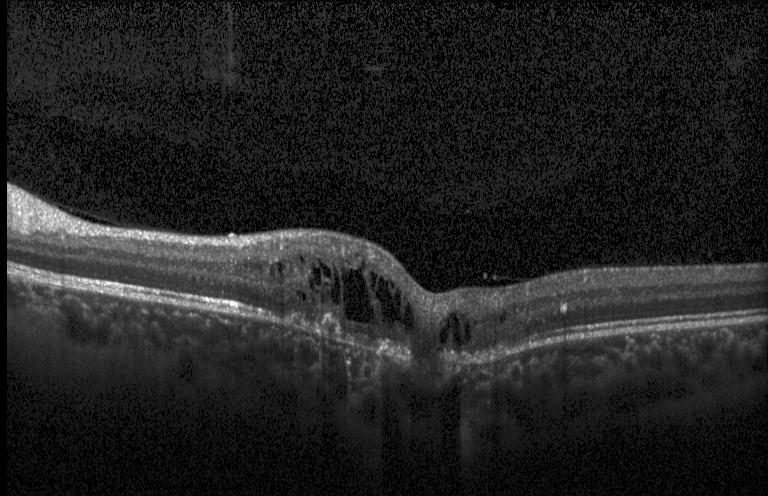
Spectral-domain optical coherence tomography. Retinal OCT cross-section. Through the macula.
Finding: a choroidal neovascular membrane.